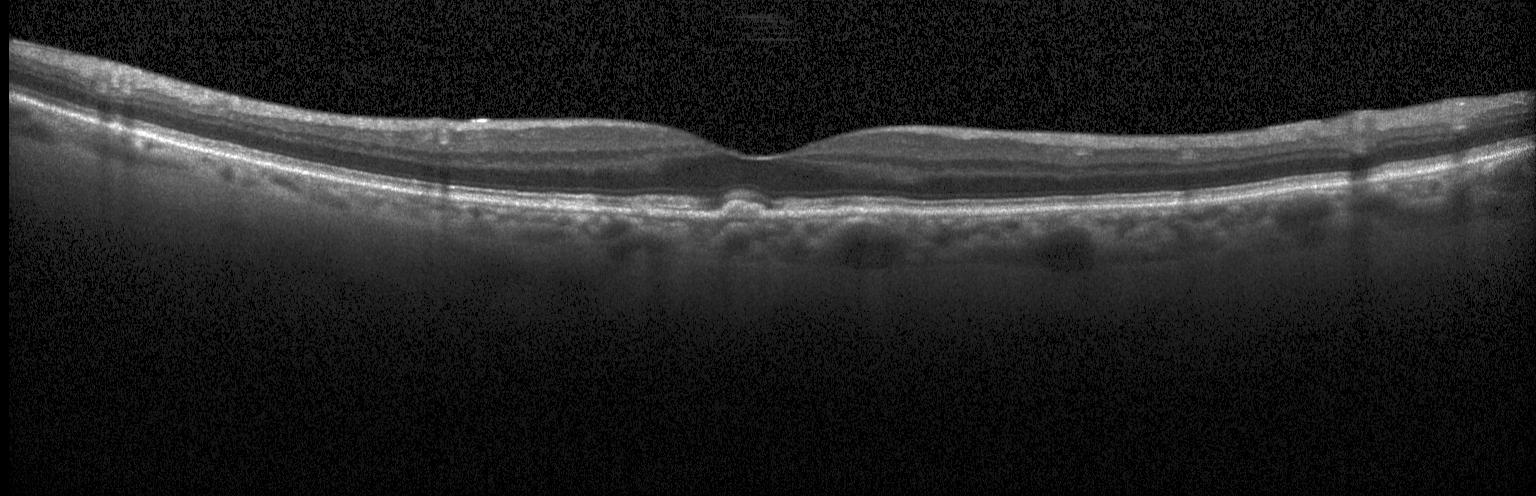

Heidelberg Spectralis. Through the macula. Retinal OCT B-scan — Assessment: drusen.